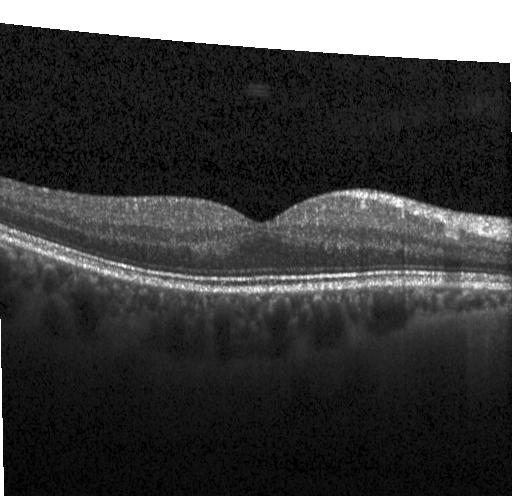
Finding: no choroidal neovascularization, no diabetic macular edema, and no drusen.